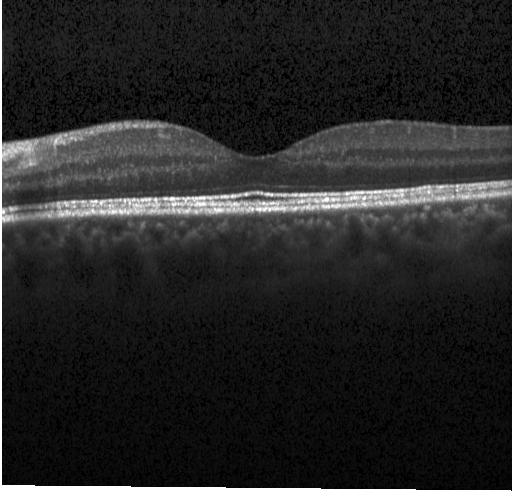

SD-OCT; optical coherence tomography B-scan. Diagnosis: no choroidal neovascularization, diabetic macular edema, or drusen.